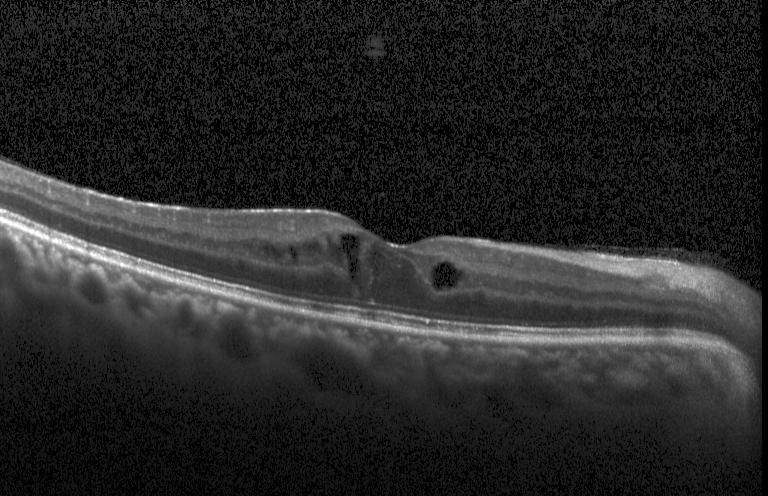

Diagnosis: diabetic macular edema.